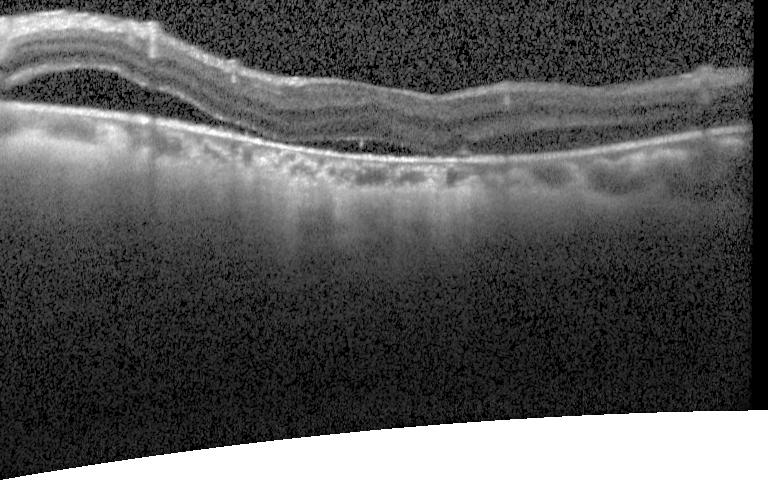
OCT B-scan
The scan shows a choroidal neovascular membrane.